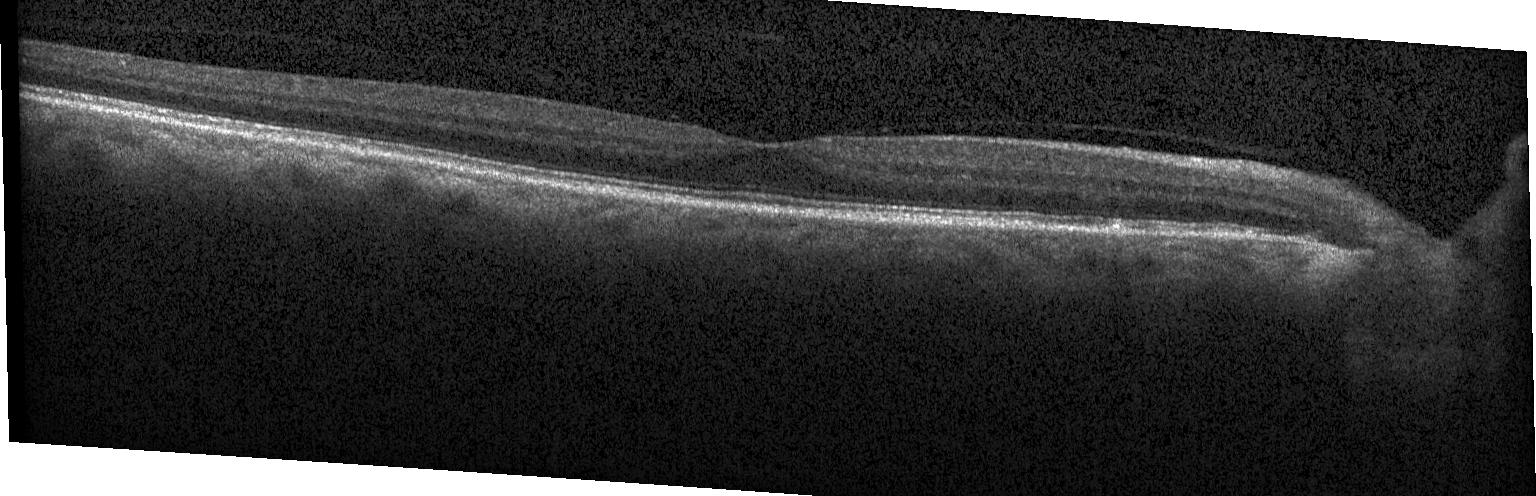 No choroidal neovascularization, no diabetic macular edema, and no drusen.